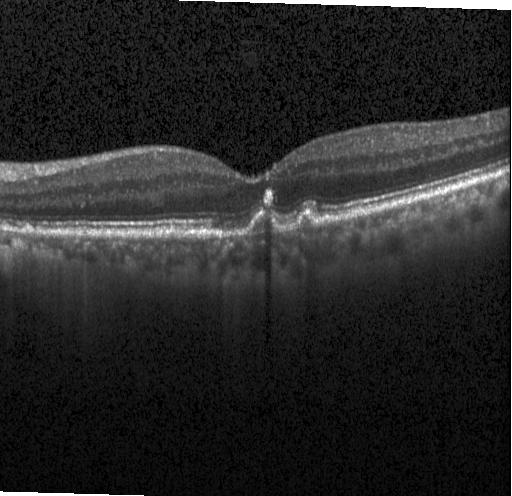 Retinal OCT cross-section, SD-OCT
Dx: multiple drusen.